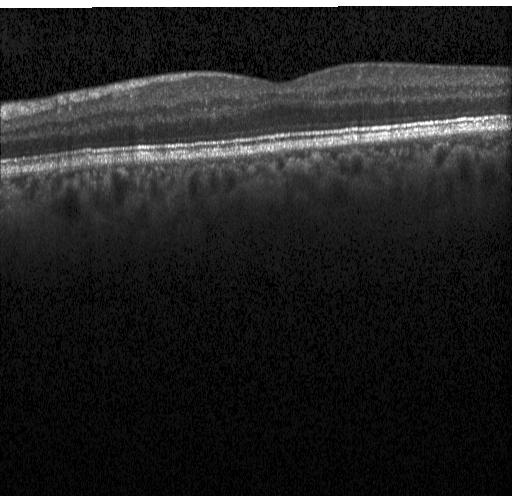 OCT finding: no evidence of choroidal neovascularization, diabetic macular edema, or drusen.